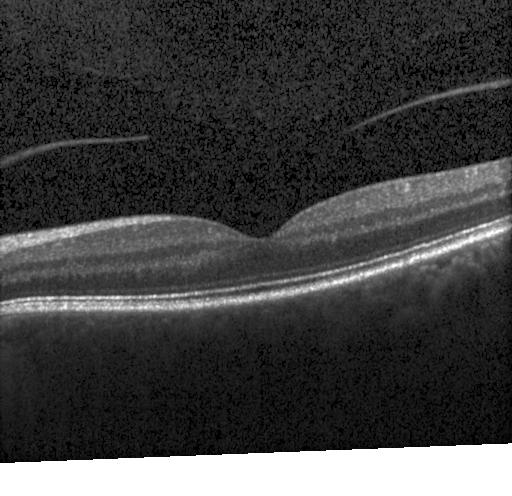

SD-OCT; optical coherence tomography B-scan. OCT finding: no choroidal neovascularization, diabetic macular edema, or drusen.